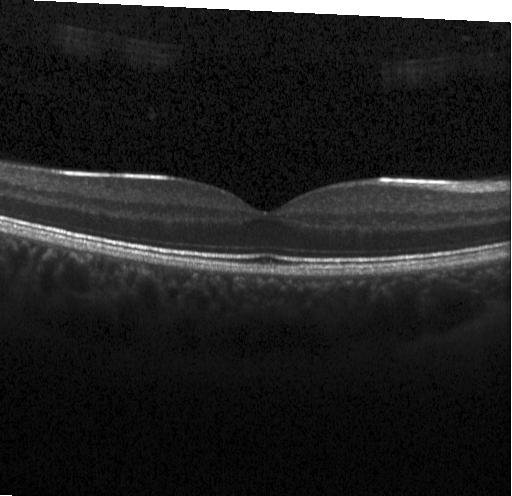 Heidelberg Spectralis. Optical coherence tomography B-scan. Spectral-domain optical coherence tomography. The scan shows neither CNV, DME, nor drusen.